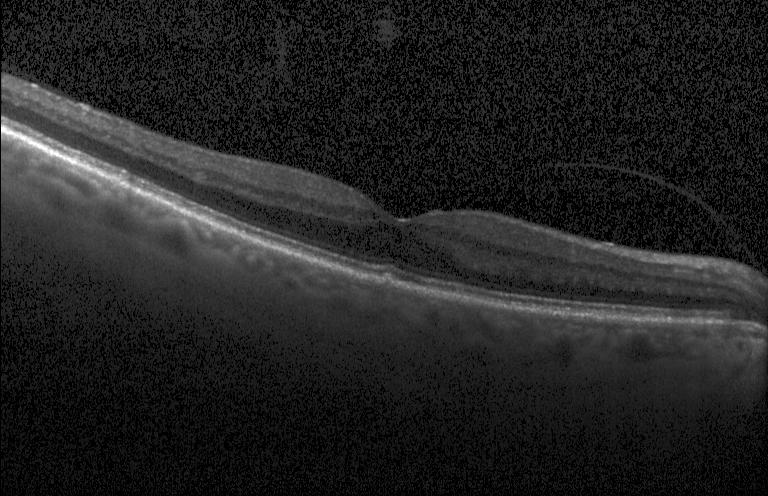 Acquired on a Heidelberg Spectralis. Through the macula. Spectral-domain OCT. Optical coherence tomography B-scan
Impression: no choroidal neovascularization, diabetic macular edema, or drusen.